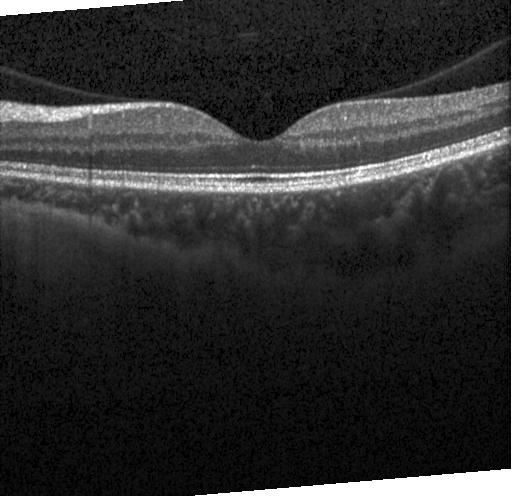
Heidelberg Spectralis. Retinal OCT B-scan. Horizontal scan through the fovea. Spectral-domain OCT.
Diagnosis: neither choroidal neovascularization, diabetic macular edema, nor drusen.